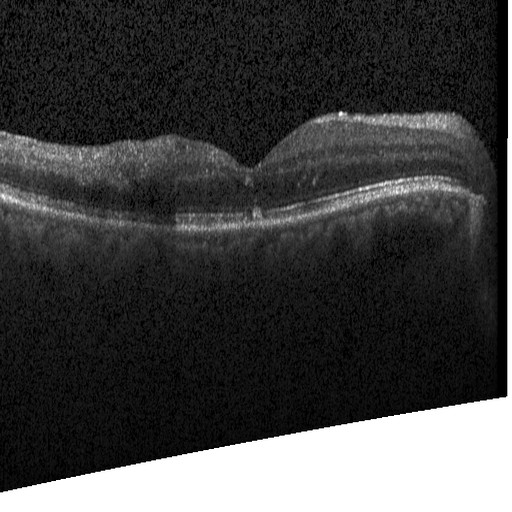 Assessment: diabetic macular edema.